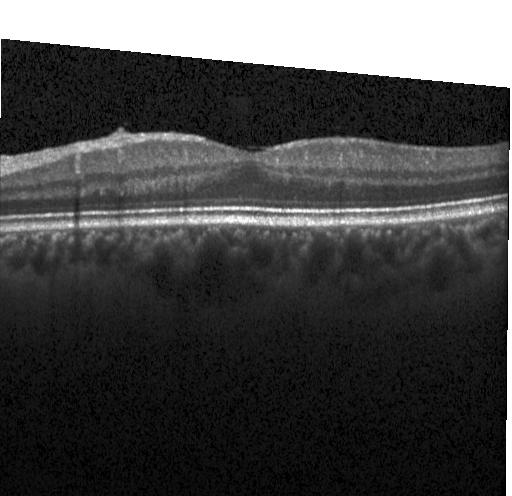

Retinal OCT cross-section.
Finding: neither choroidal neovascularization, diabetic macular edema, nor drusen.